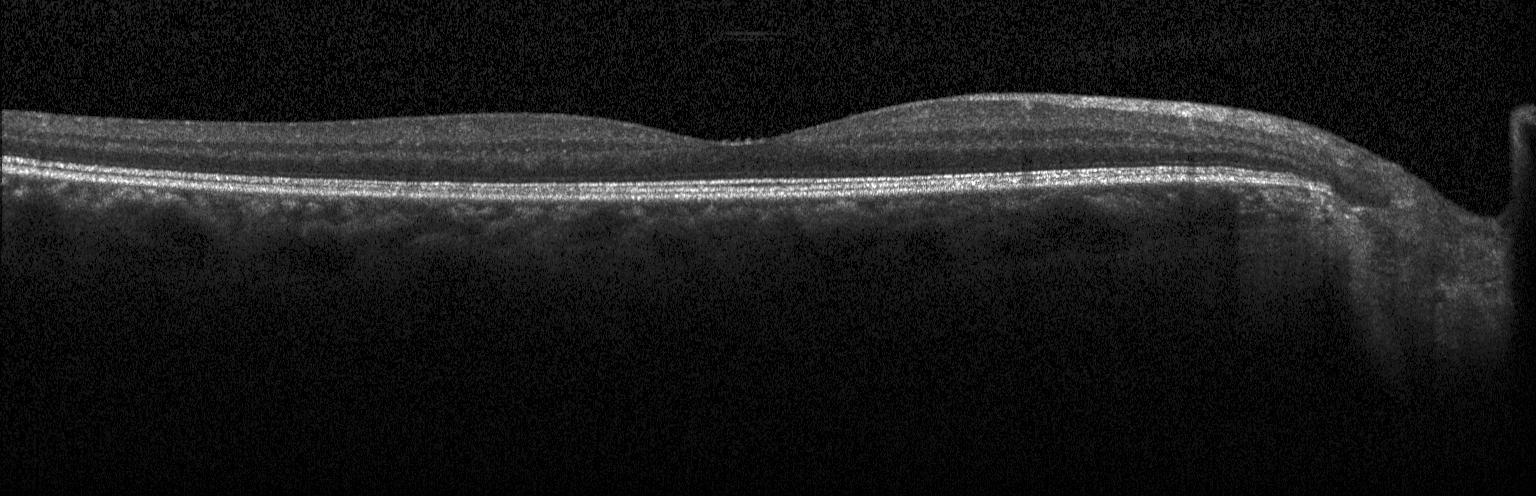
OCT line scan. Horizontal scan through the fovea — Neither choroidal neovascularization, diabetic macular edema, nor drusen.